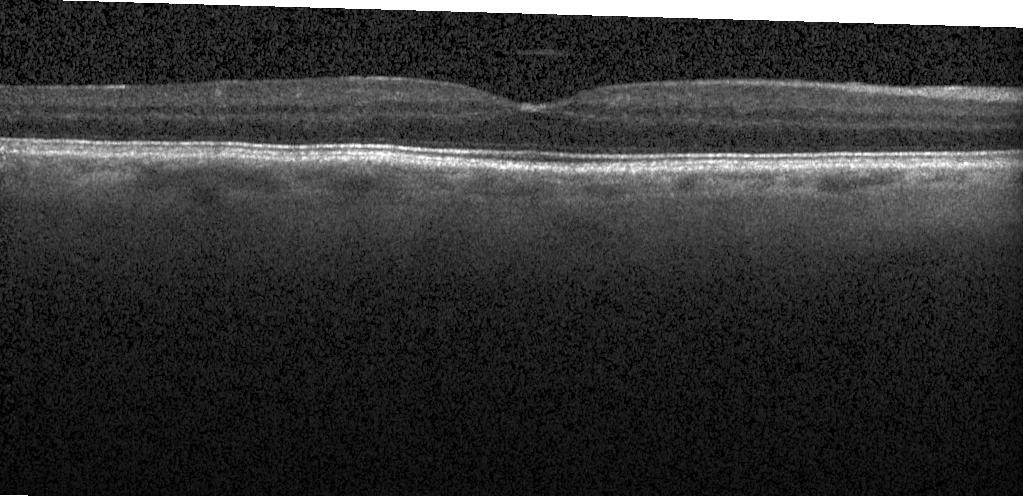
Horizontal scan through the fovea. Instrument: Heidelberg Spectralis. OCT B-scan — Finding: no choroidal neovascularization, no diabetic macular edema, and no drusen.